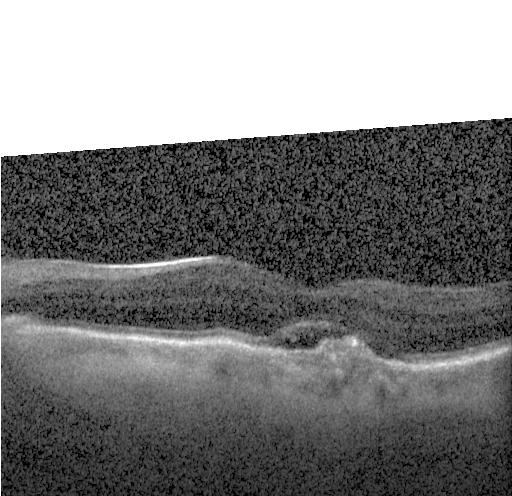

OCT B-scan showing a choroidal neovascular membrane.